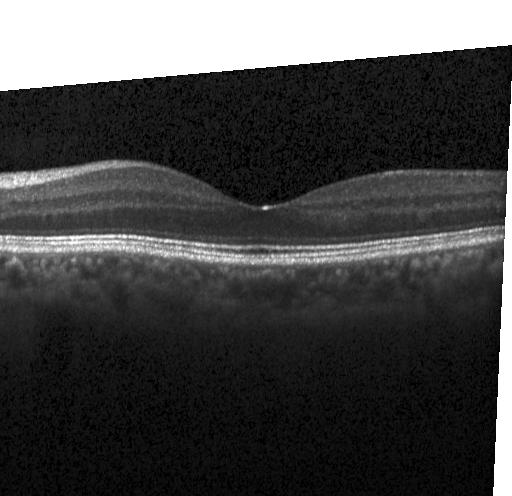
Finding: no choroidal neovascularization, no diabetic macular edema, and no drusen.